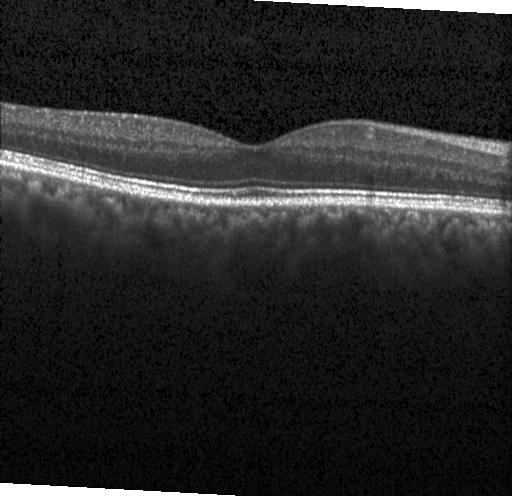
Finding: no evidence of choroidal neovascularization, diabetic macular edema, or drusen.